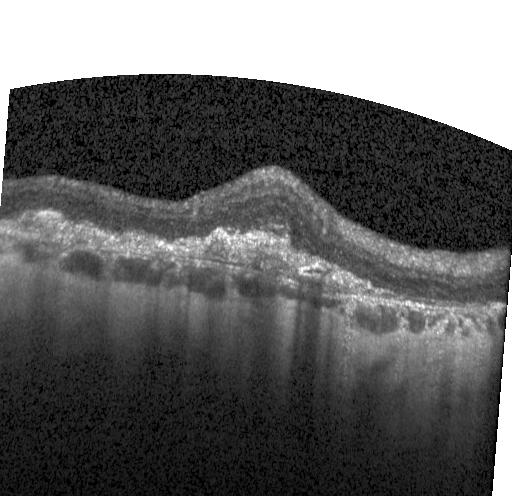

Macular scan; optical coherence tomography B-scan
Diagnosis: CNV.